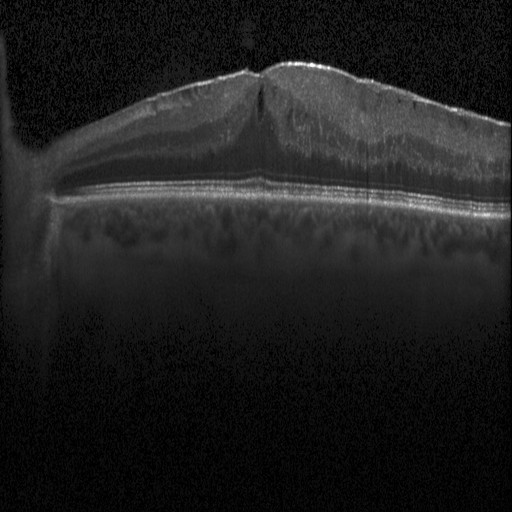
Finding: diabetic macular edema.